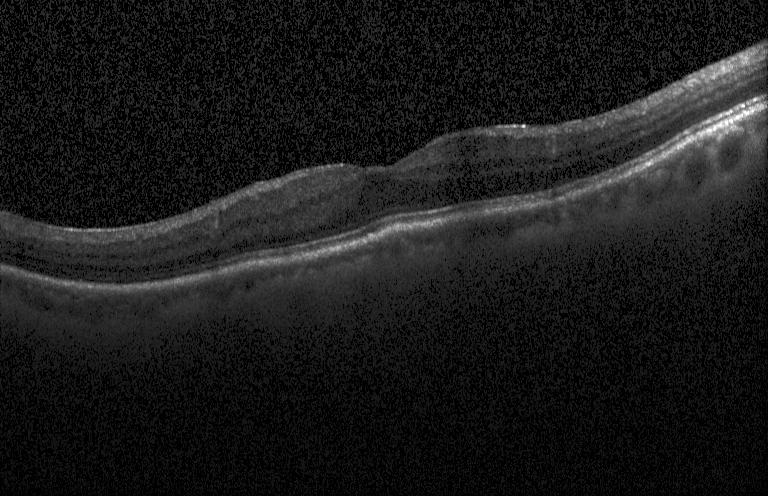
OCT B-scan. Dx: no evidence of CNV, DME, or drusen.